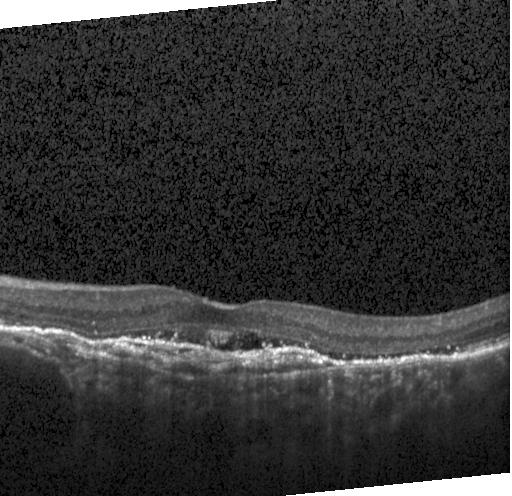

Optical coherence tomography B-scan — Finding: choroidal neovascularization.